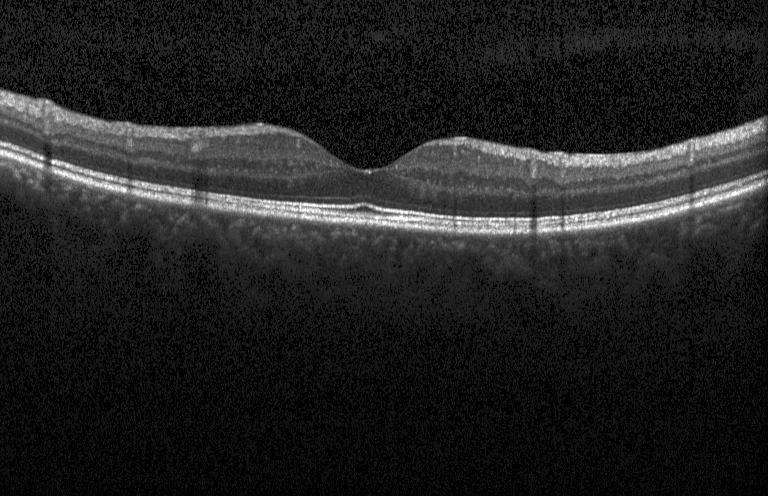

Retinal OCT cross-section. Heidelberg Spectralis. Centered on the fovea
Assessment: no choroidal neovascularization, no diabetic macular edema, and no drusen.